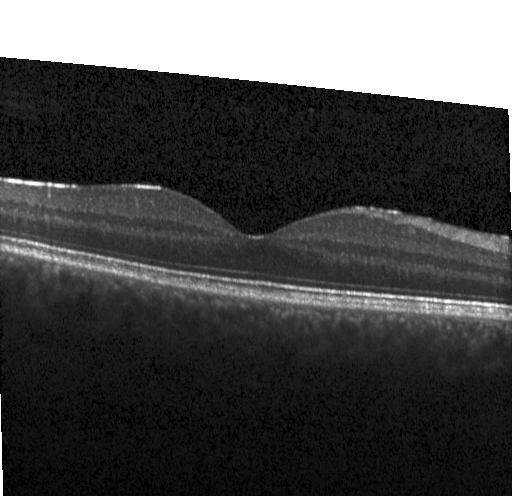

OCT B-scan · Heidelberg Spectralis
OCT finding: neither choroidal neovascularization, diabetic macular edema, nor drusen.